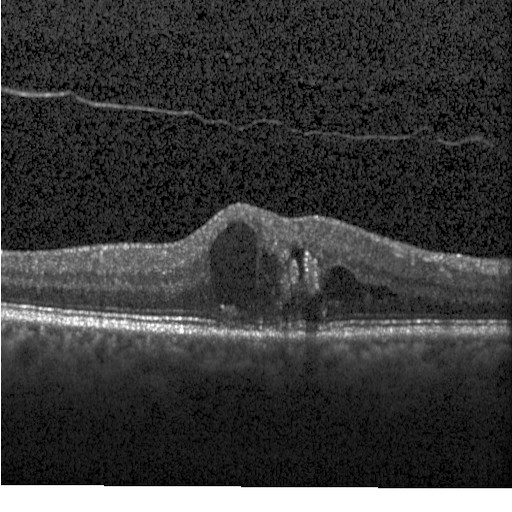 Finding: DME.